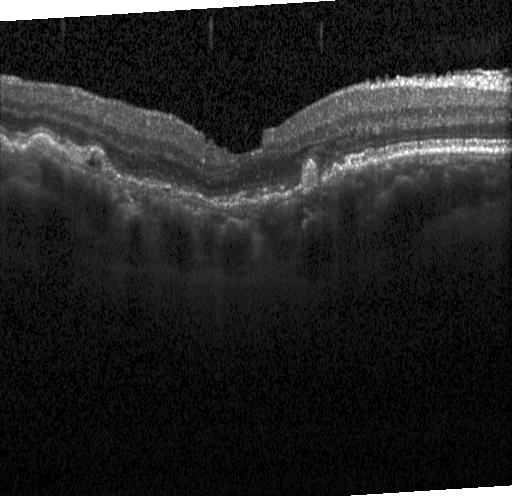 OCT line scan. Impression: a choroidal neovascular membrane.